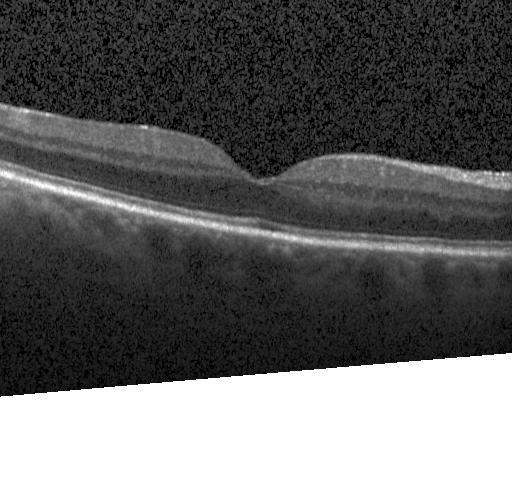

Optical coherence tomography B-scan. SD-OCT. Instrument: Heidelberg Spectralis. Fovea-centered — No CNV, no DME, and no drusen.